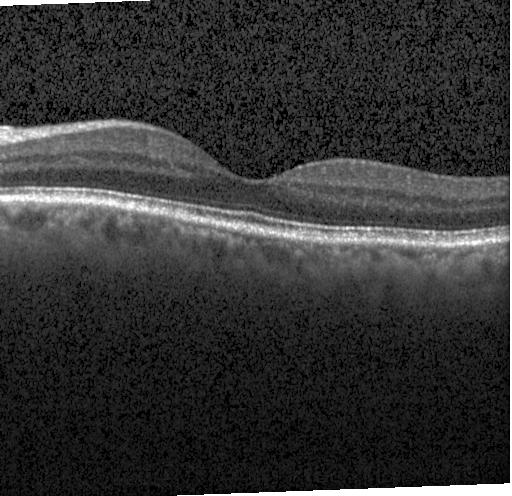

Assessment: no choroidal neovascularization, diabetic macular edema, or drusen.